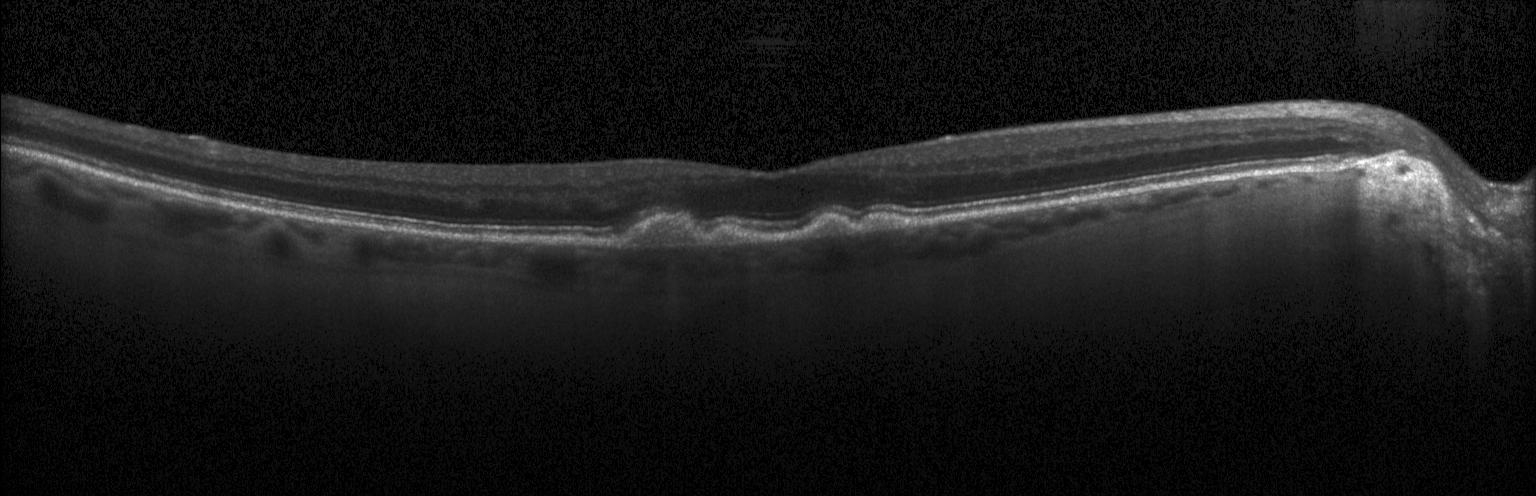 Heidelberg Spectralis; optical coherence tomography scan.
Dx: multiple drusen.